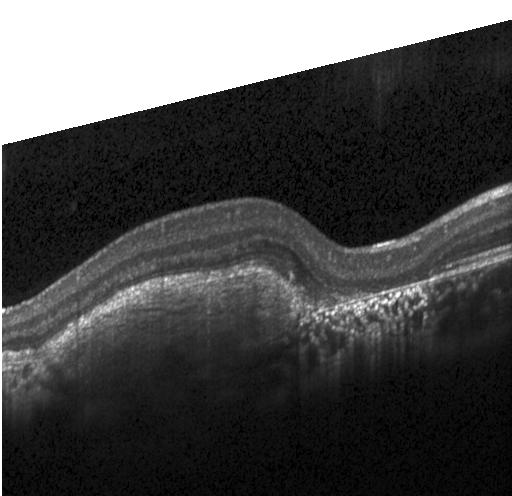 This B-scan demonstrates choroidal neovascularization.